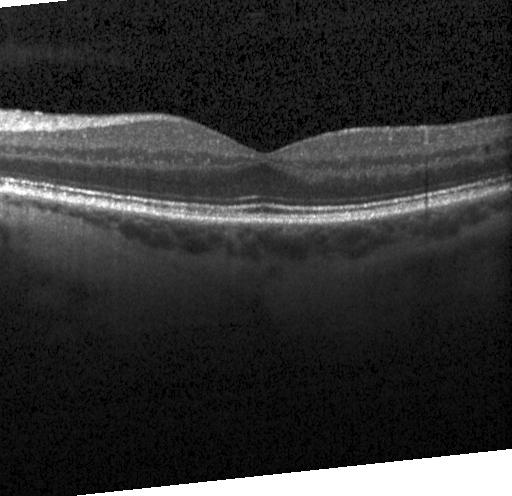 Spectral-domain OCT. Heidelberg Spectralis OCT system. Centered on the fovea. OCT B-scan
OCT finding: no evidence of choroidal neovascularization, diabetic macular edema, or drusen.